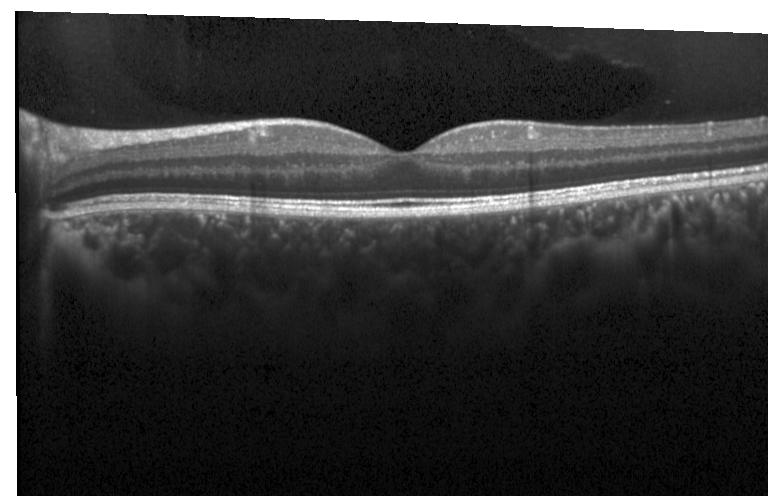

Diagnosis: no evidence of choroidal neovascularization, diabetic macular edema, or drusen.